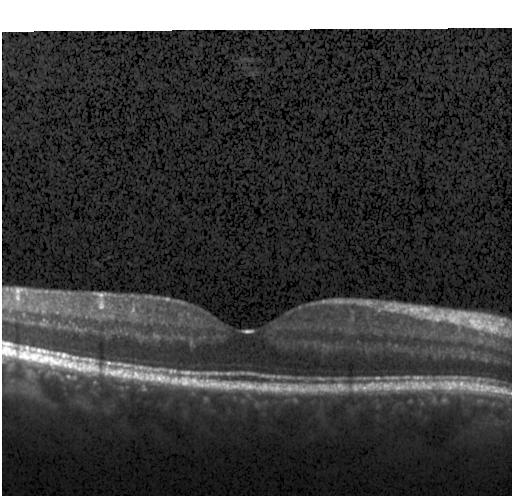 Finding: no choroidal neovascularization, diabetic macular edema, or drusen.